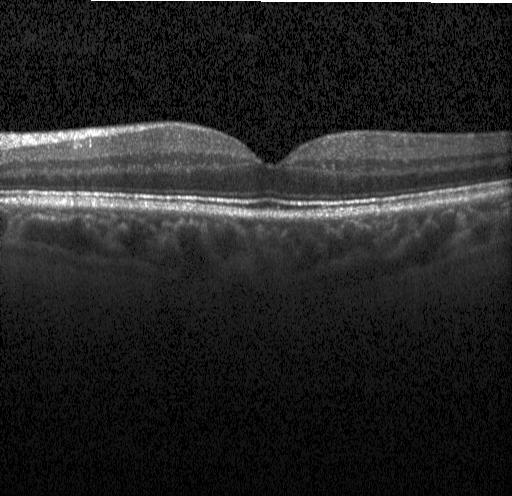 Heidelberg Spectralis · SD-OCT · retinal OCT B-scan — No CNV, no DME, and no drusen.